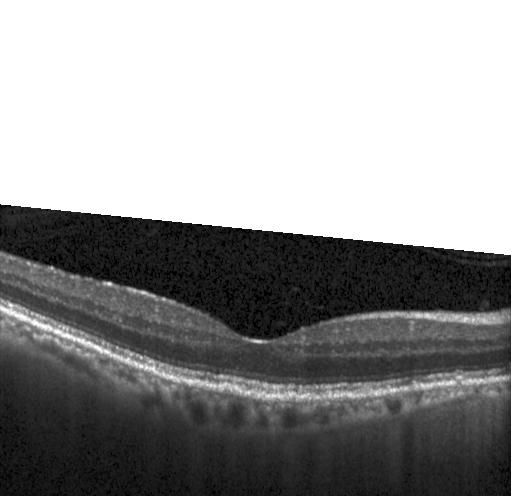
Retinal OCT B-scan — Finding: no choroidal neovascularization, no diabetic macular edema, and no drusen.